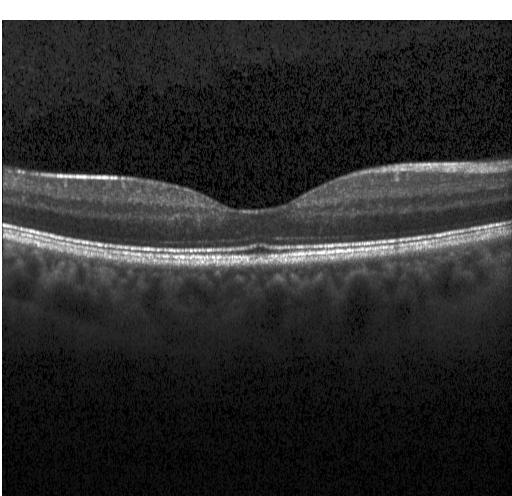 SD-OCT; macular scan; Heidelberg Spectralis OCT system; optical coherence tomography B-scan
Impression: neither choroidal neovascularization, diabetic macular edema, nor drusen.